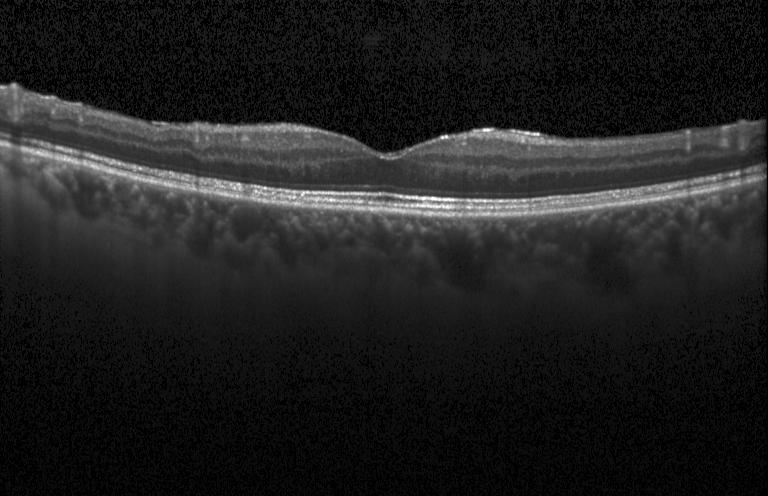 Macular scan; acquired on a Heidelberg Spectralis; spectral-domain optical coherence tomography; OCT B-scan. Diagnosis: no evidence of choroidal neovascularization, diabetic macular edema, or drusen.